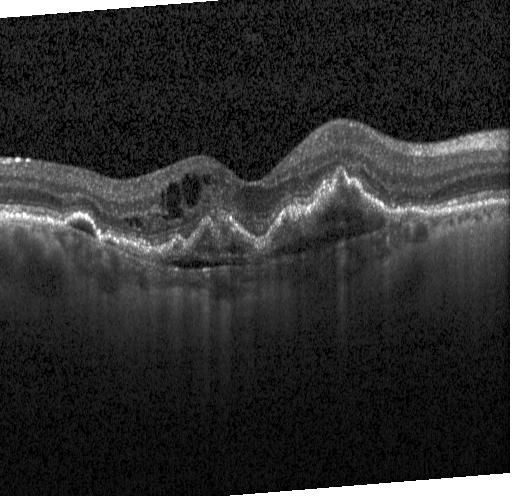 OCT B-scan showing choroidal neovascularization.